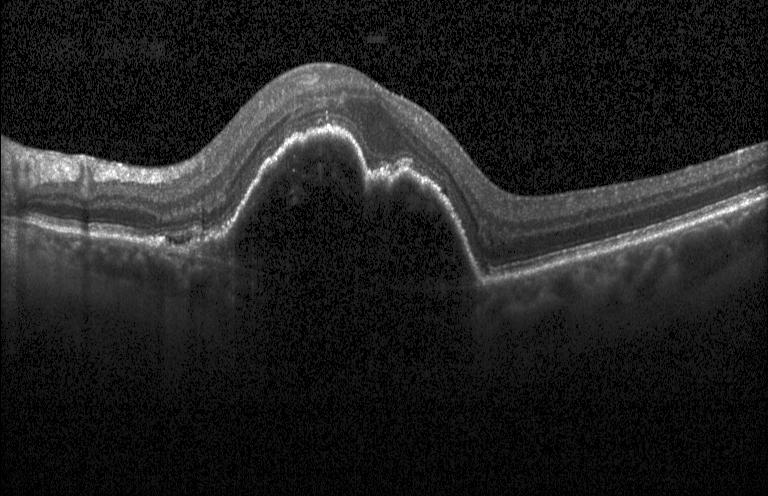
Finding: a choroidal neovascular membrane.